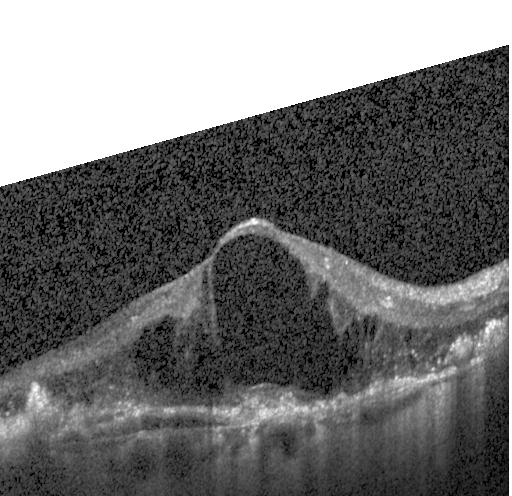 Instrument: Heidelberg Spectralis. Optical coherence tomography B-scan.
CNV.